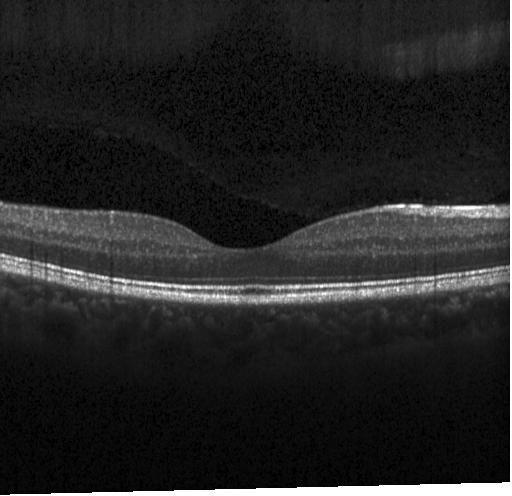 The scan shows no evidence of choroidal neovascularization, diabetic macular edema, or drusen.